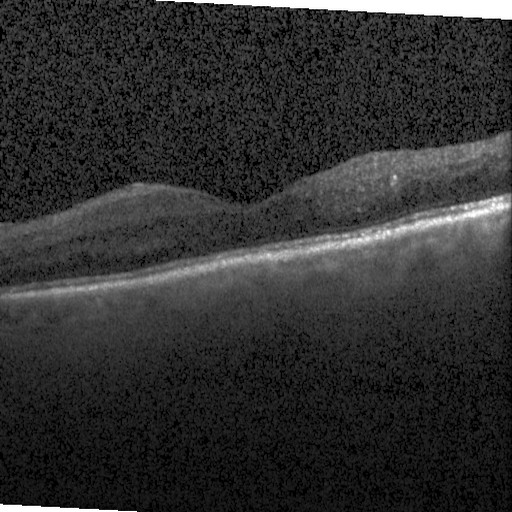

OCT line scan · acquired on a Heidelberg Spectralis · through the macula
Diabetic macular edema.